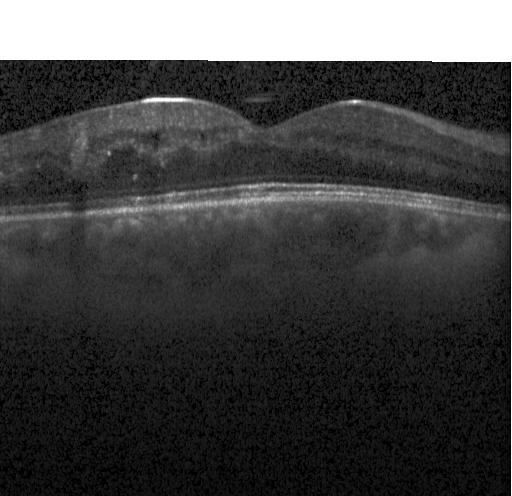

Optical coherence tomography scan; instrument: Heidelberg Spectralis.
Macular OCT: diabetic macular edema.